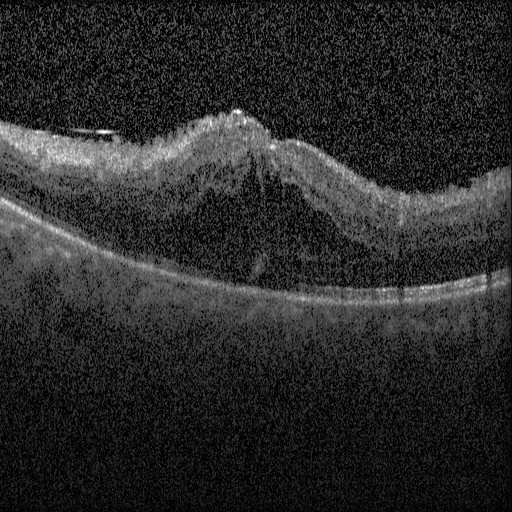 Optical coherence tomography scan. Macular OCT: diabetic macular edema.